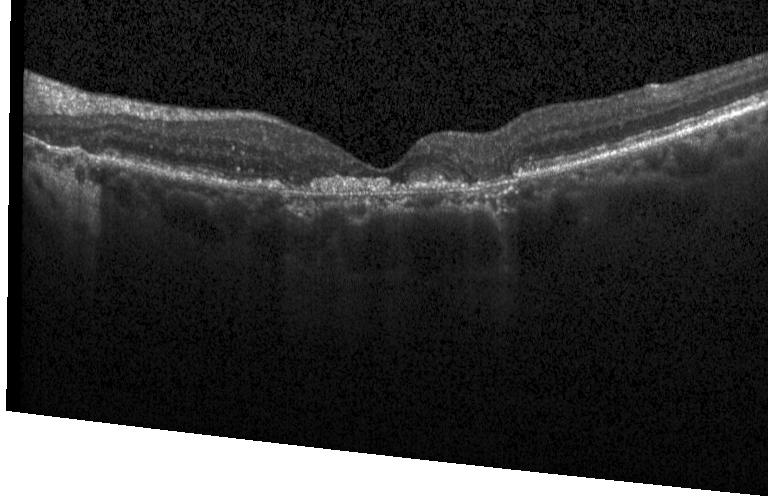 OCT line scan
The scan shows CNV.